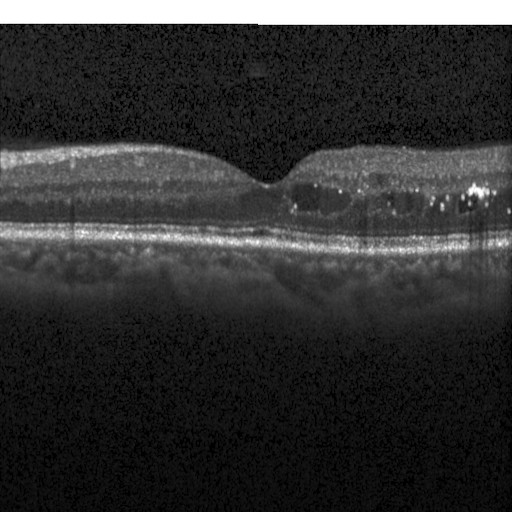 Spectral-domain OCT, OCT line scan. Diagnosis: diabetic macular edema.